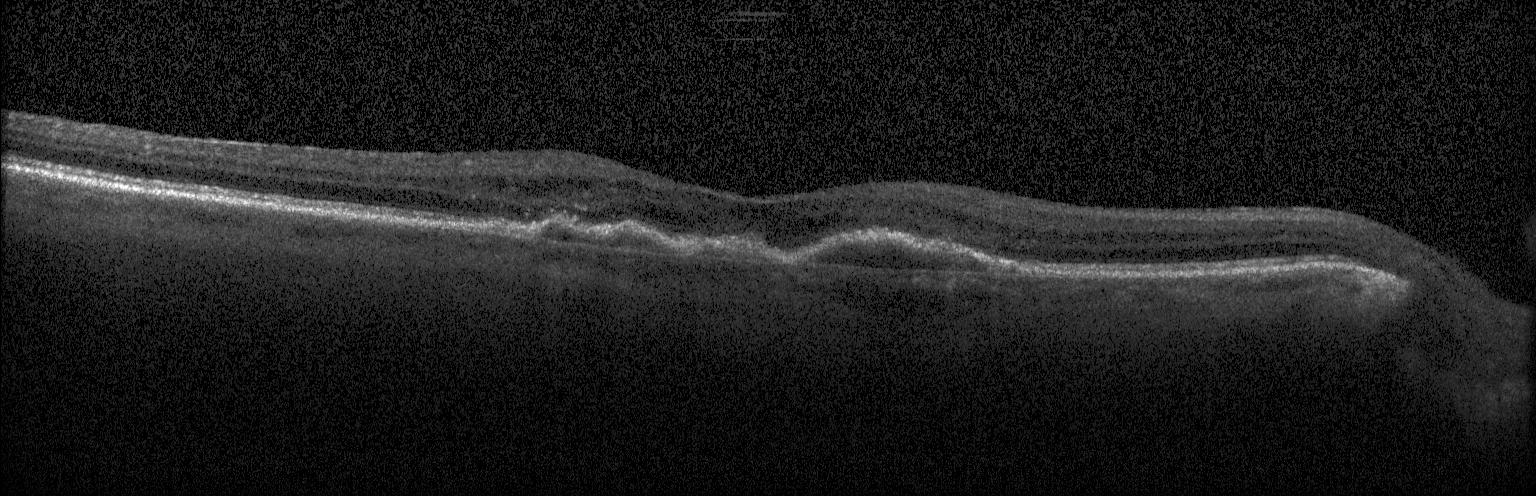
Spectral-domain optical coherence tomography, retinal OCT B-scan, through the macula — Finding: a choroidal neovascular membrane.